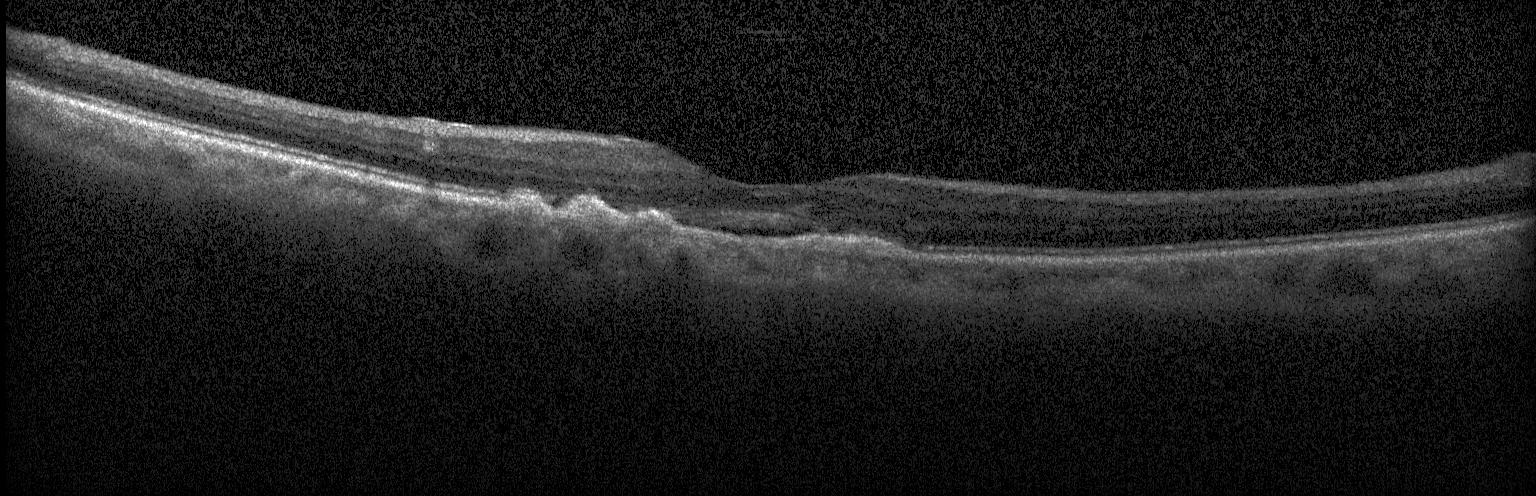
Spectral-domain OCT · optical coherence tomography scan · through the macula · instrument: Heidelberg Spectralis — CNV.